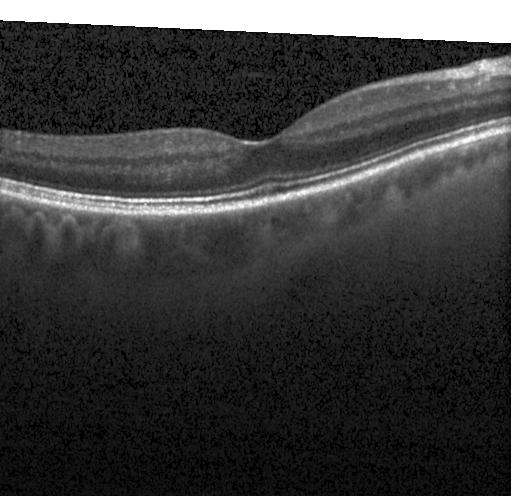

OCT B-scan showing no evidence of CNV, DME, or drusen.